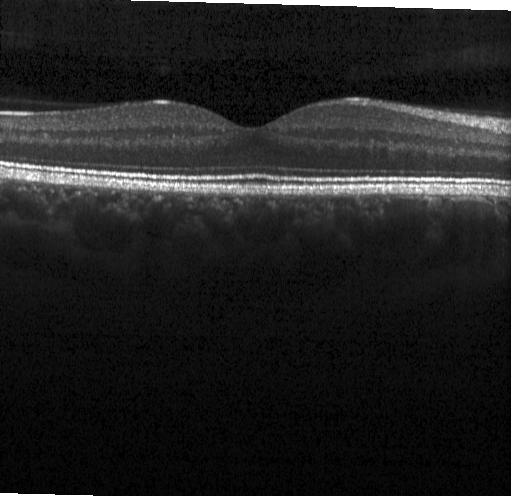

Spectral-domain OCT B-scan: no CNV, no DME, and no drusen.